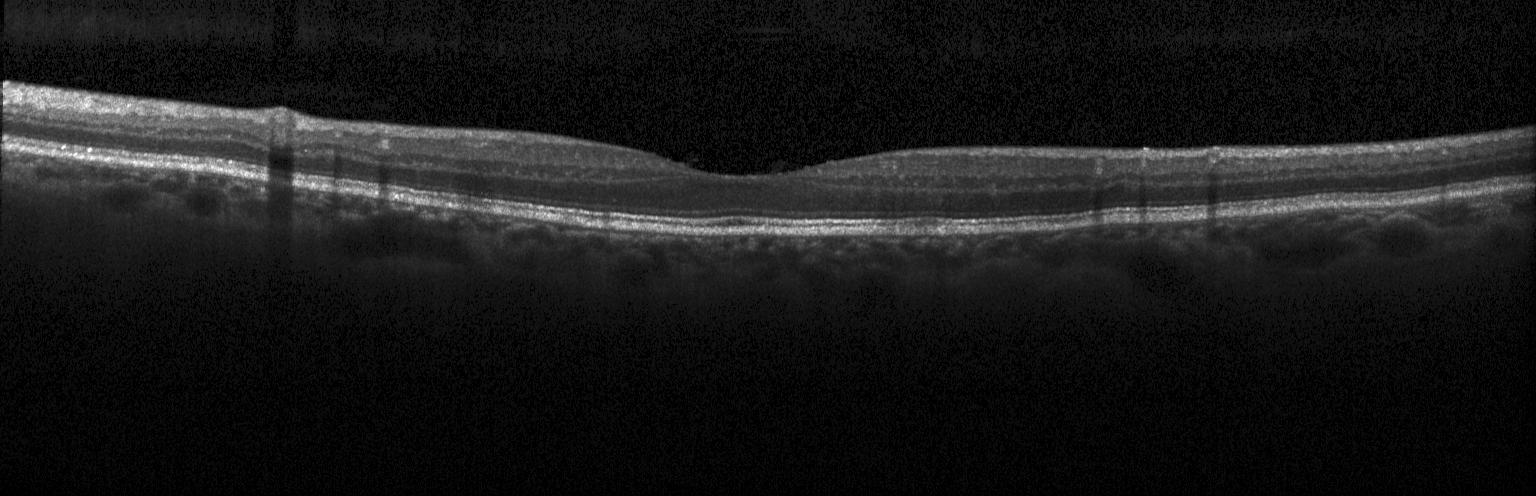

Acquired on a Heidelberg Spectralis, SD-OCT, OCT line scan, through the macula.
This B-scan demonstrates neither choroidal neovascularization, diabetic macular edema, nor drusen.